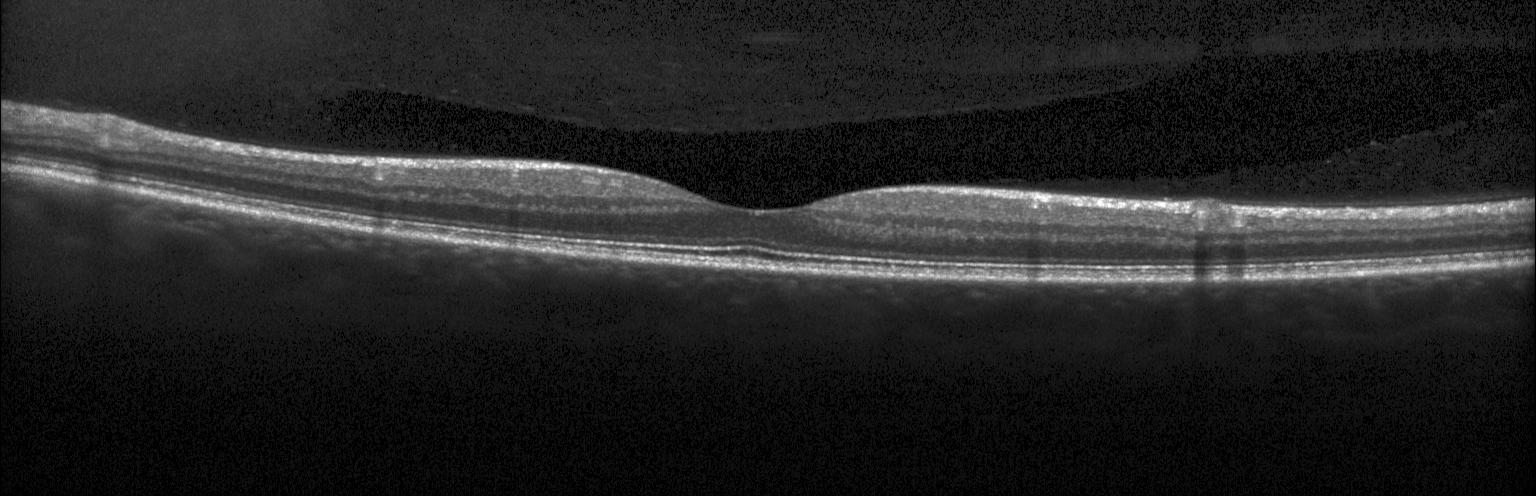
OCT line scan. Finding: neither choroidal neovascularization, diabetic macular edema, nor drusen.